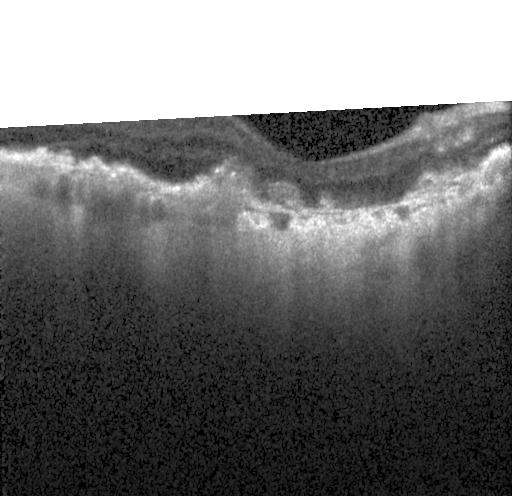

Macular OCT: a choroidal neovascular membrane.